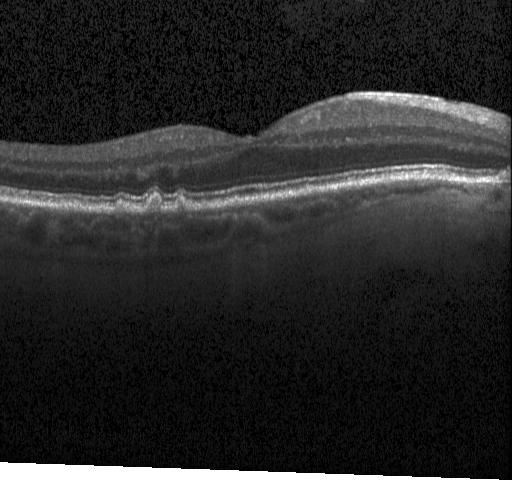

Fovea-centered · OCT B-scan · spectral-domain OCT. Macular OCT: multiple drusen.